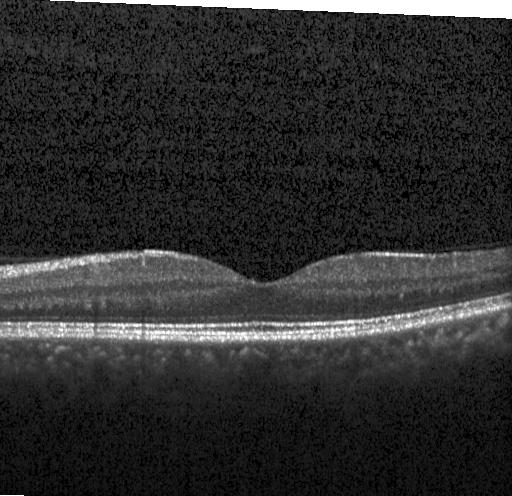 Spectral-domain OCT · OCT B-scan · acquired on a Heidelberg Spectralis · through the macula.
Assessment: no choroidal neovascularization, no diabetic macular edema, and no drusen.